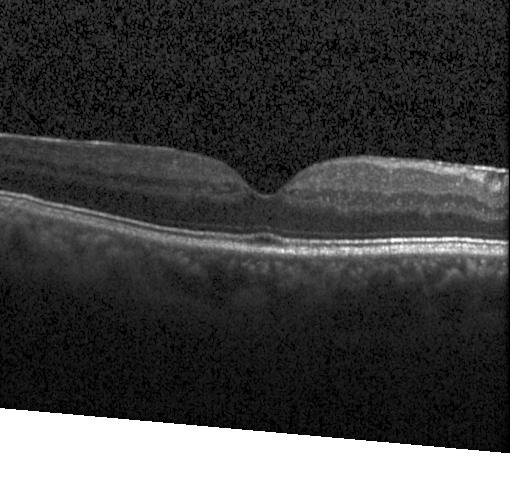

Dx: no evidence of choroidal neovascularization, diabetic macular edema, or drusen.